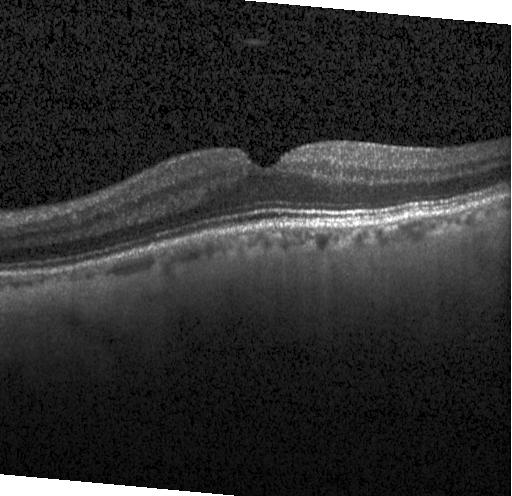
OCT finding: no CNV, DME, or drusen.